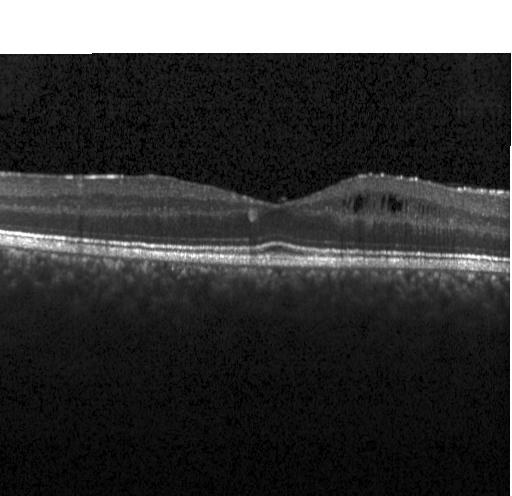

The scan shows diabetic macular edema.